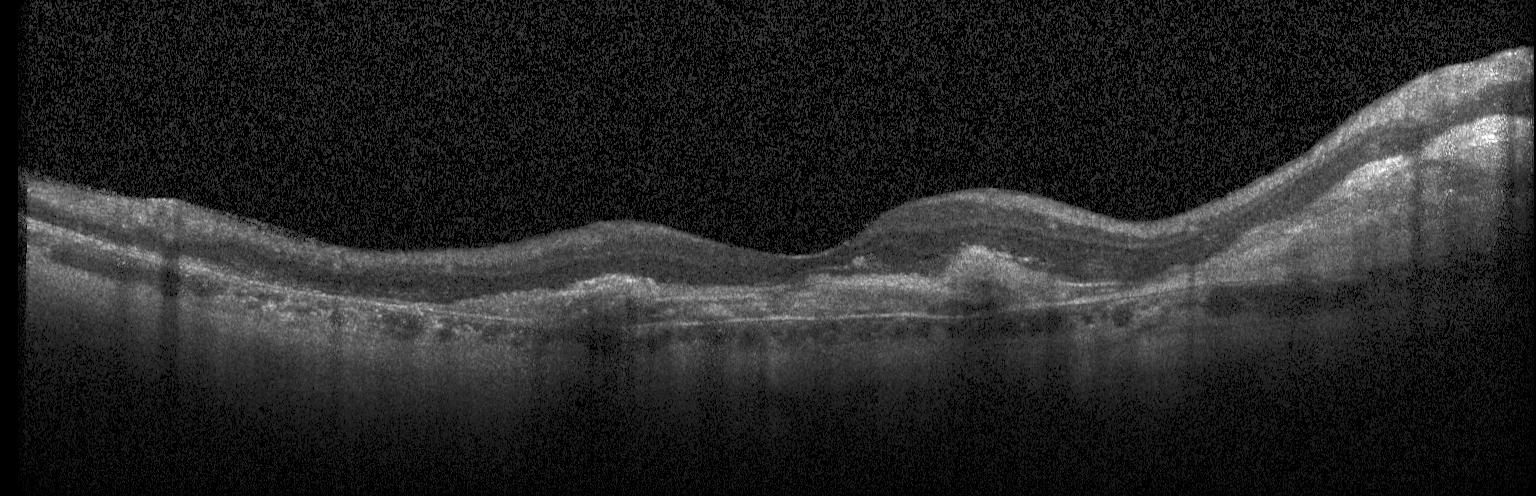

Through the macula; retinal OCT B-scan; spectral-domain OCT; Heidelberg Spectralis
OCT finding: choroidal neovascularization (CNV).